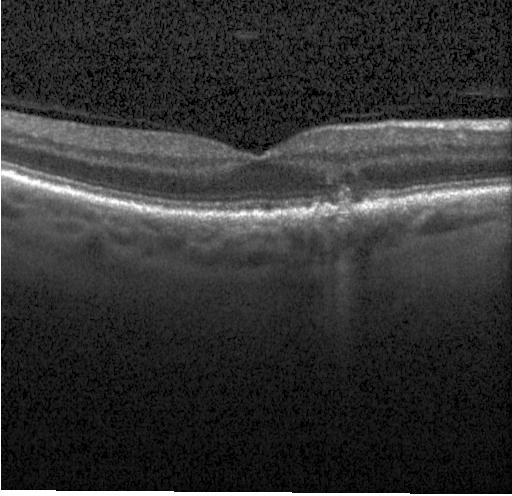 Optical coherence tomography B-scan · spectral-domain optical coherence tomography
Drusen.